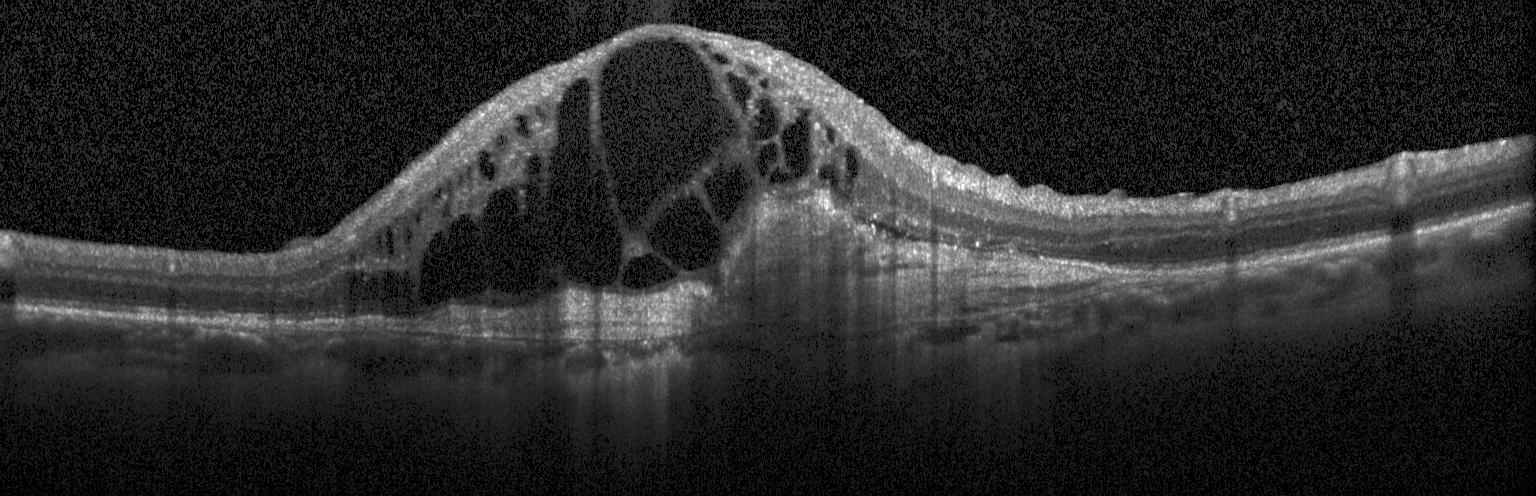 Assessment: choroidal neovascularization.